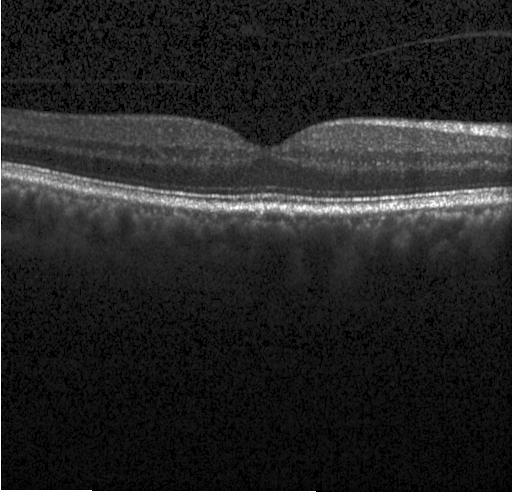 Optical coherence tomography B-scan. Macular OCT: no CNV, no DME, and no drusen.